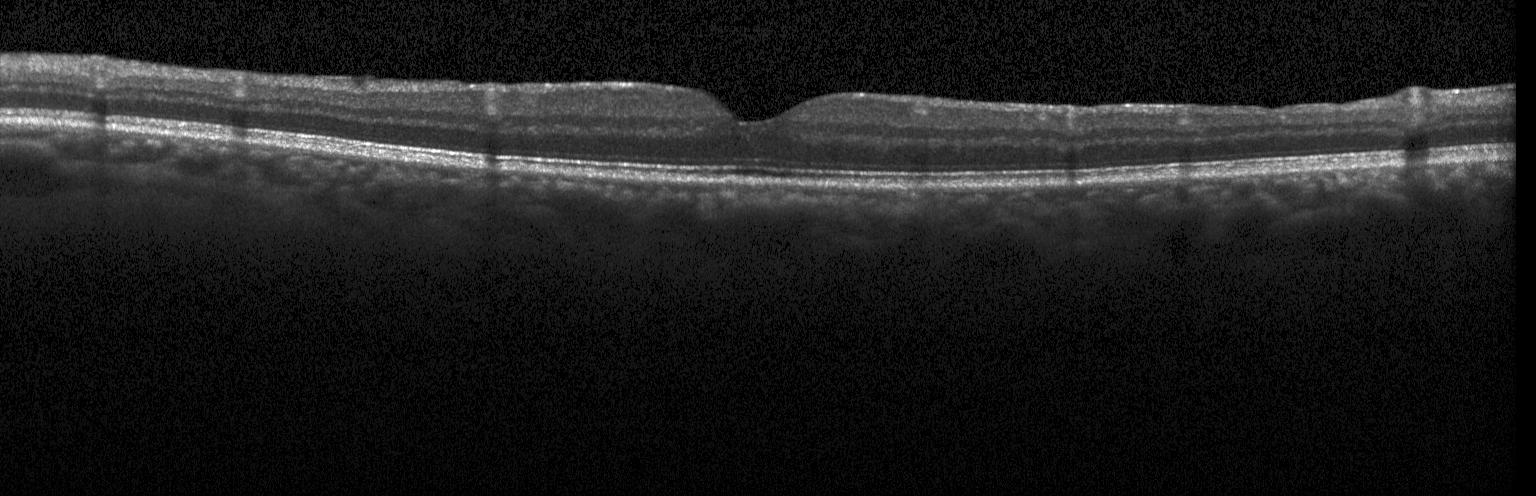

OCT scan showing no evidence of CNV, DME, or drusen.